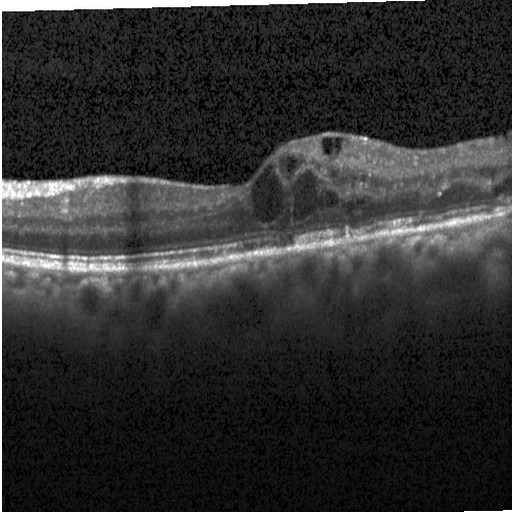 Fovea-centered; spectral-domain OCT; acquired on a Heidelberg Spectralis; OCT B-scan.
Finding: diabetic macular edema.